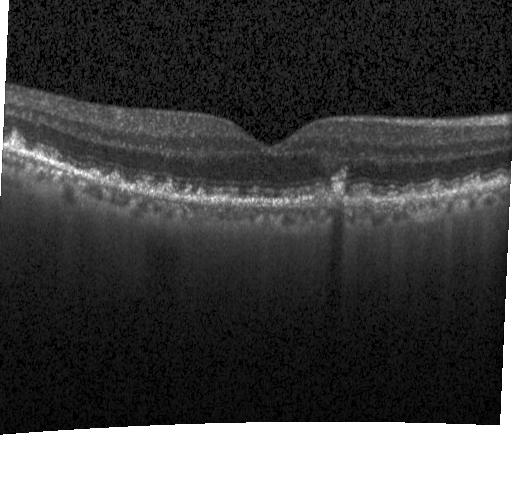

OCT B-scan · through the macula. Diagnosis: drusen.